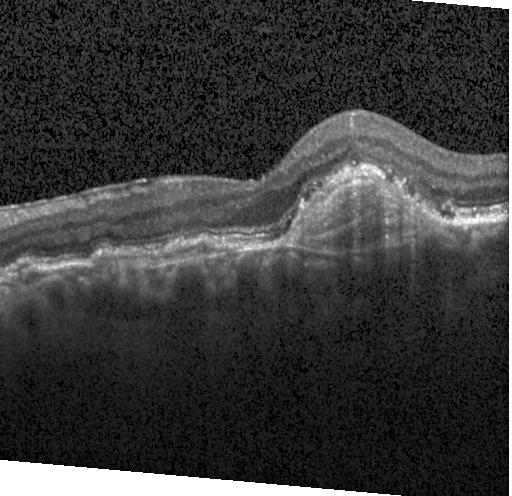

Fovea-centered. Retinal OCT cross-section — Assessment: a choroidal neovascular membrane.